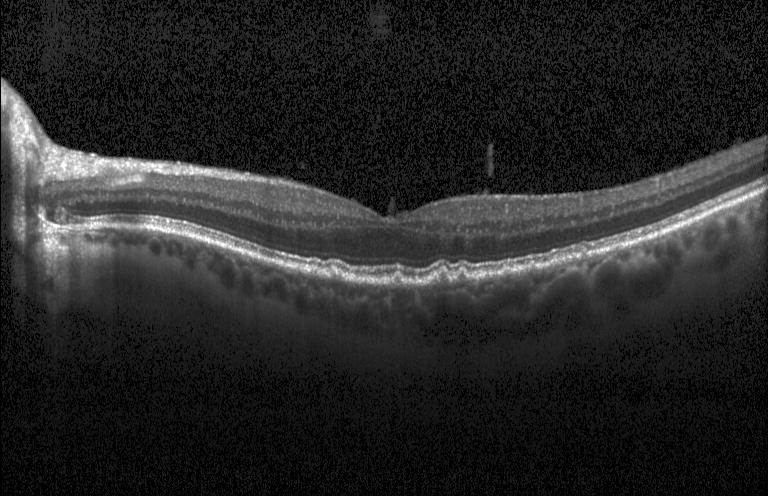 OCT B-scan
Multiple drusen.